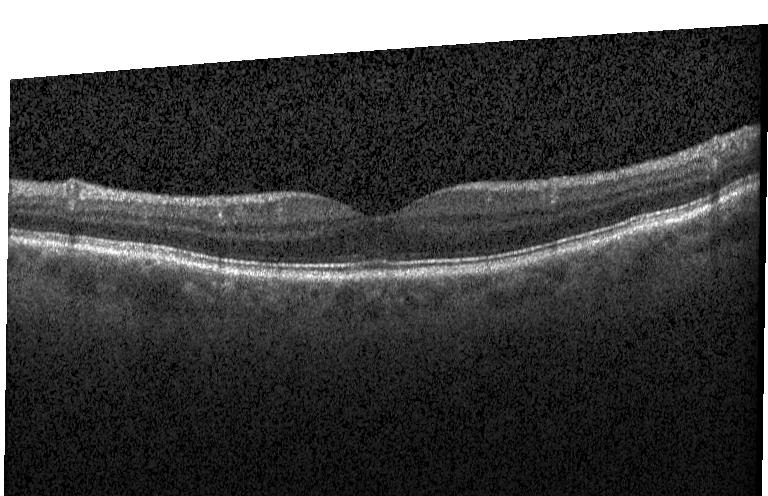

Instrument: Heidelberg Spectralis; optical coherence tomography B-scan — This B-scan demonstrates neither choroidal neovascularization, diabetic macular edema, nor drusen.